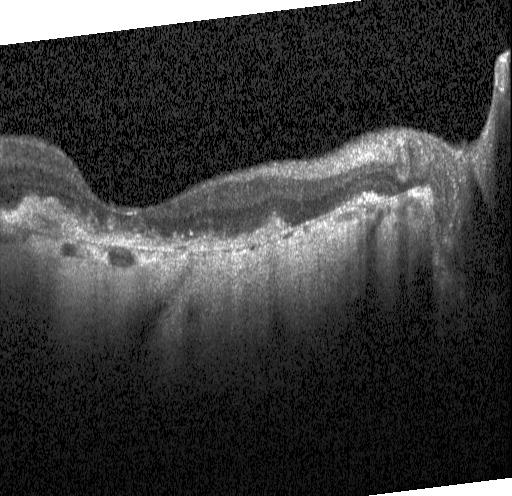
Macular OCT: choroidal neovascularization.